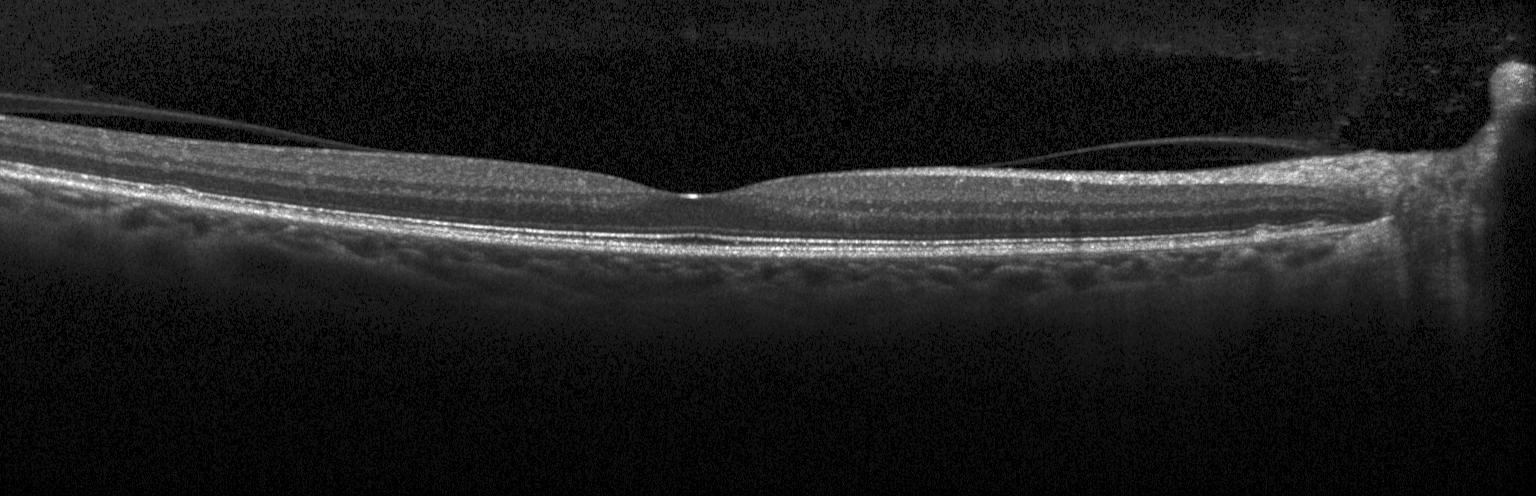 Retinal OCT B-scan. Impression: no choroidal neovascularization, diabetic macular edema, or drusen.